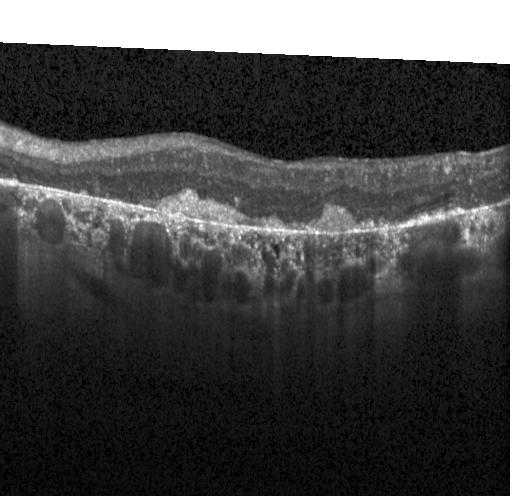 OCT line scan, instrument: Heidelberg Spectralis
Choroidal neovascularization.